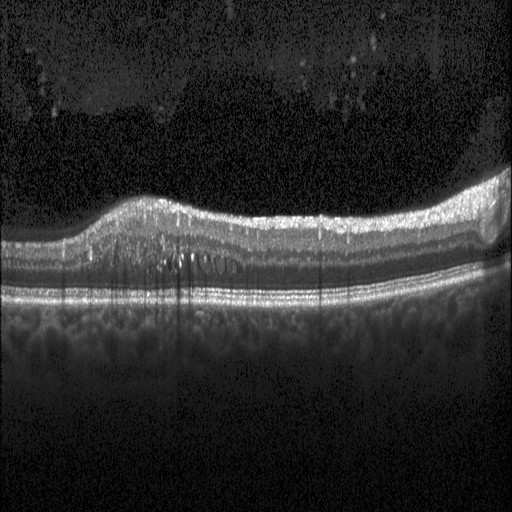

Diagnosis: diabetic macular edema.